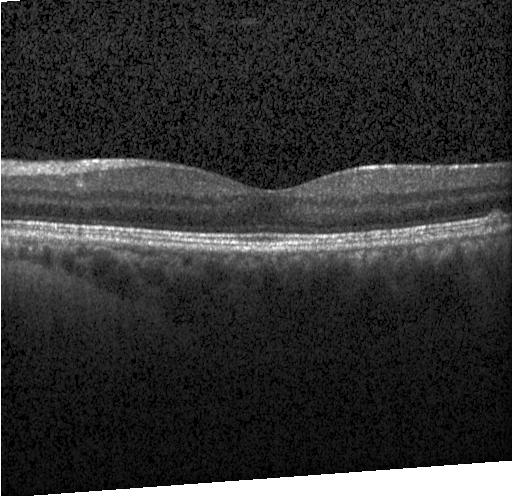 OCT line scan. Sub-RPE drusenoid deposits.